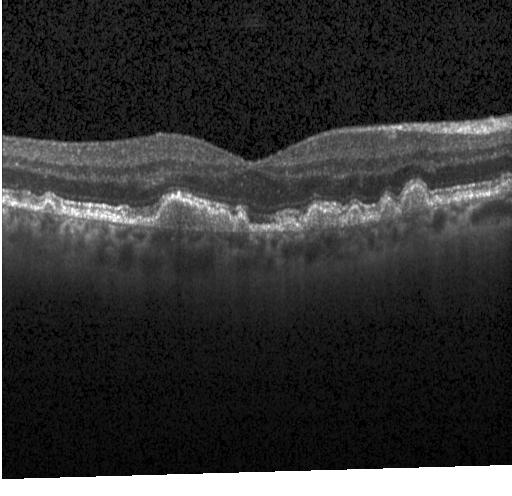

Dx: sub-RPE drusenoid deposits.